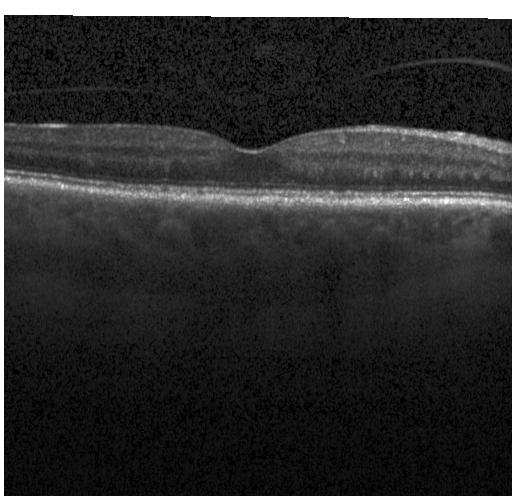
Optical coherence tomography scan — Assessment: no choroidal neovascularization, diabetic macular edema, or drusen.